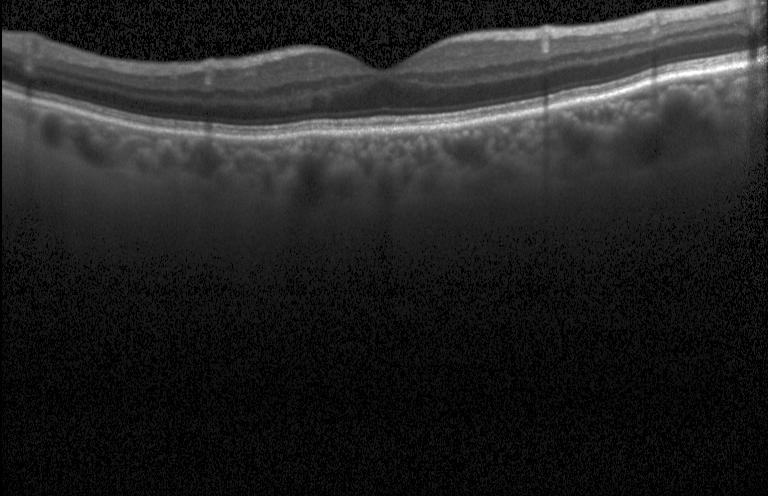
Diagnosis: no choroidal neovascularization, no diabetic macular edema, and no drusen.